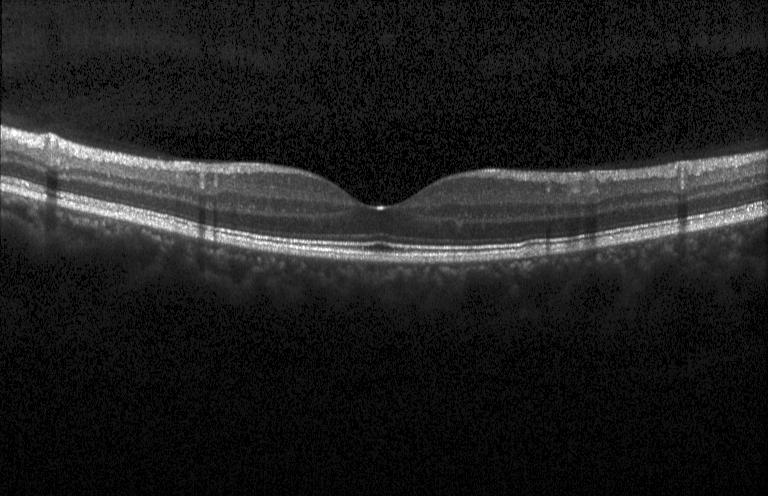 Diagnosis: no evidence of choroidal neovascularization, diabetic macular edema, or drusen.